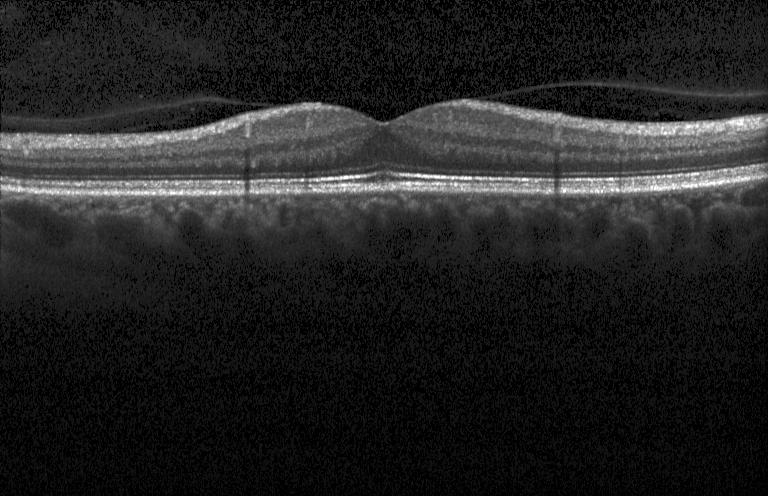 Optical coherence tomography B-scan, spectral-domain optical coherence tomography, Heidelberg Spectralis, through the macula
Finding: no evidence of choroidal neovascularization, diabetic macular edema, or drusen.